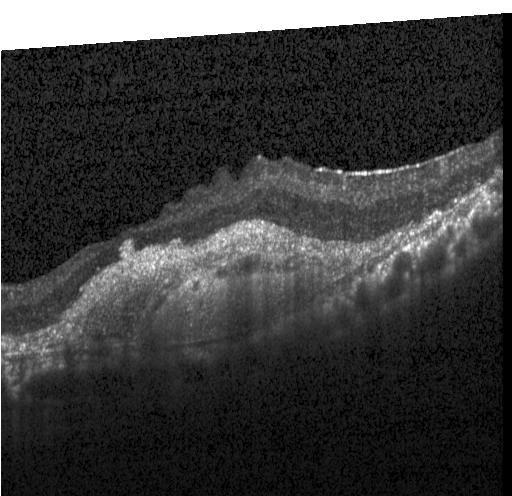

Instrument: Heidelberg Spectralis; horizontal scan through the fovea; optical coherence tomography scan; spectral-domain OCT. Finding: choroidal neovascularization.